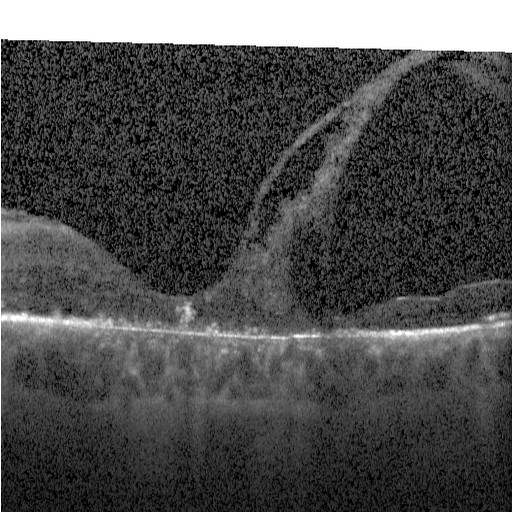

Acquired on a Heidelberg Spectralis. Spectral-domain OCT. Optical coherence tomography scan
Dx: DME.